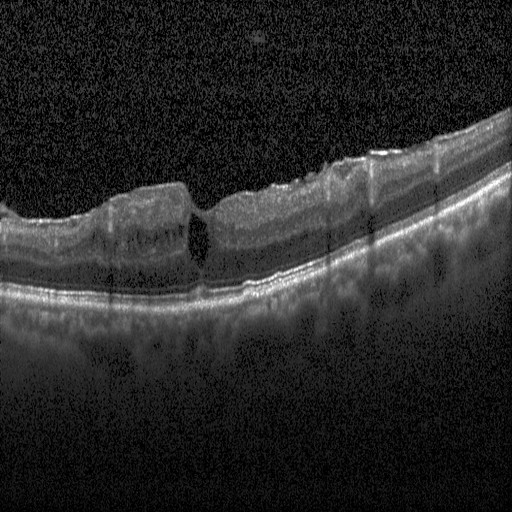
OCT B-scan. Finding: diabetic macular edema.